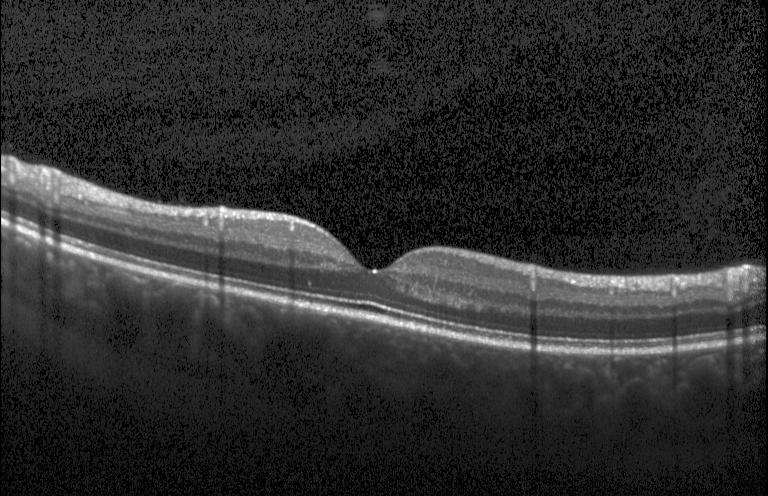
Neither CNV, DME, nor drusen.